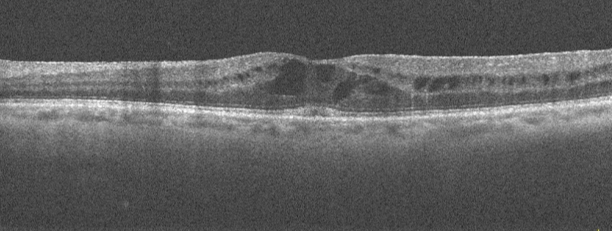
OCT line scan; fovea-centered; instrument: Optovue Avanti RTVue XR
Impression: diabetic macular edema (DME).